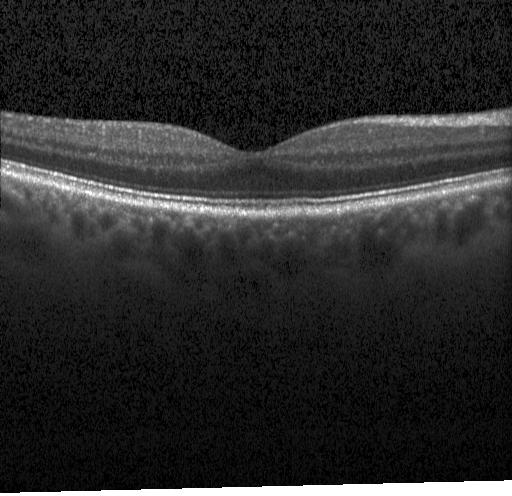 Dx: neither choroidal neovascularization, diabetic macular edema, nor drusen.